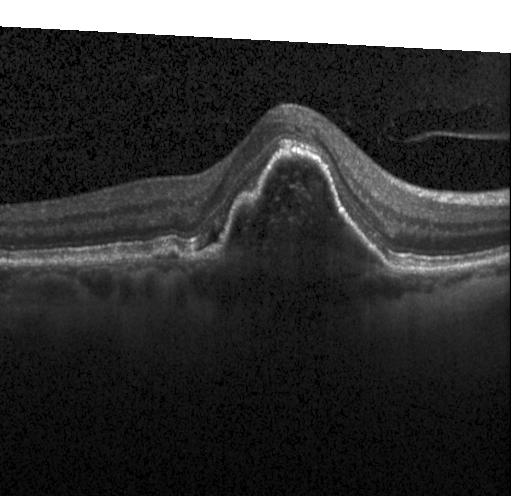
OCT B-scan. Finding: a choroidal neovascular membrane.